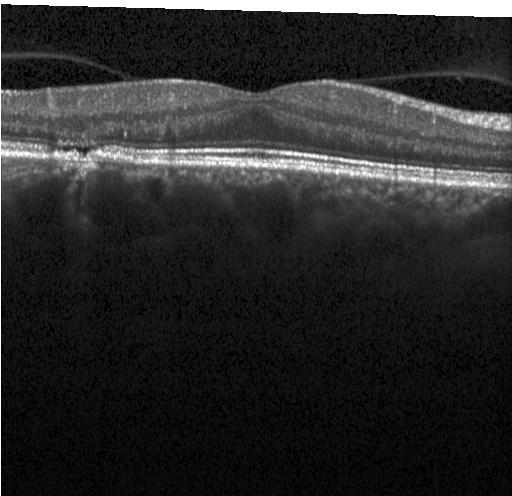
Retinal OCT B-scan.
This B-scan demonstrates a choroidal neovascular membrane.